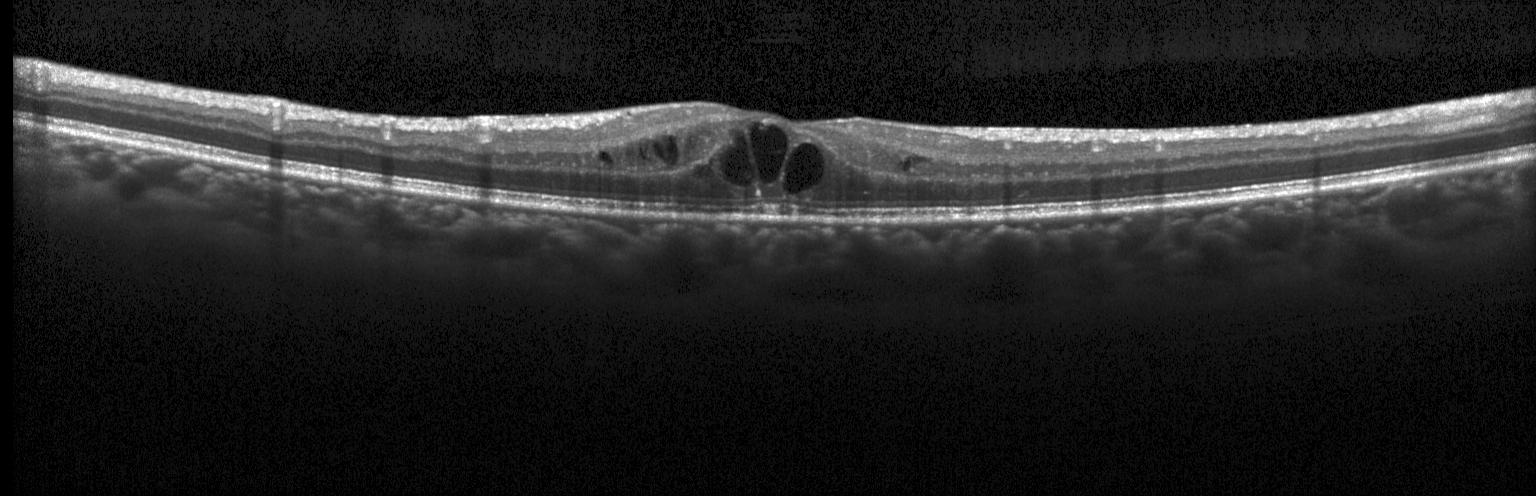 Optical coherence tomography B-scan. Diagnosis: diabetic macular edema.